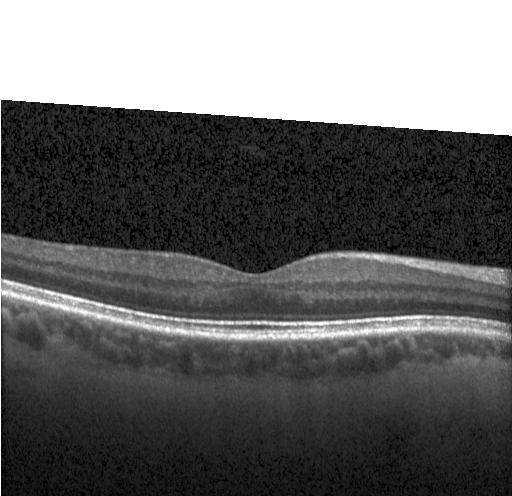 No choroidal neovascularization, diabetic macular edema, or drusen.